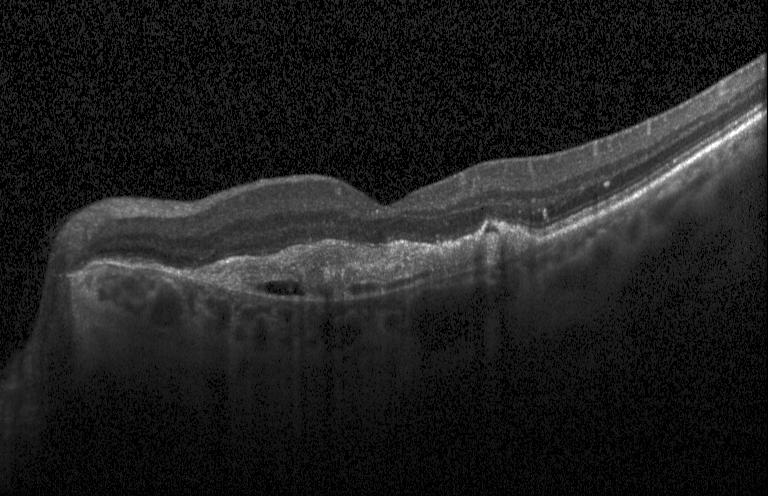
Spectral-domain OCT. Heidelberg Spectralis OCT system. Through the macula. Optical coherence tomography B-scan.
Finding: choroidal neovascularization (CNV).